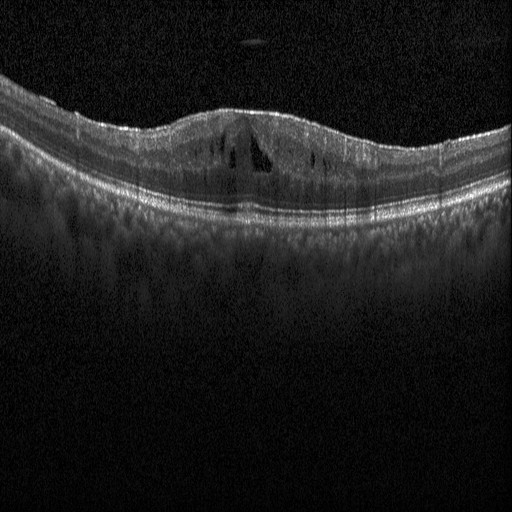

OCT B-scan. Fovea-centered — Diagnosis: DME.